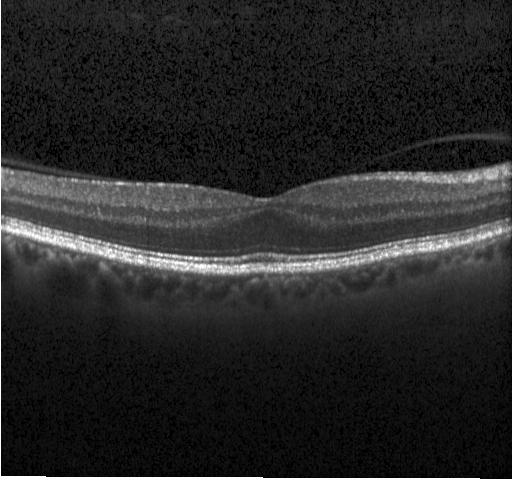

OCT finding: no choroidal neovascularization, diabetic macular edema, or drusen.